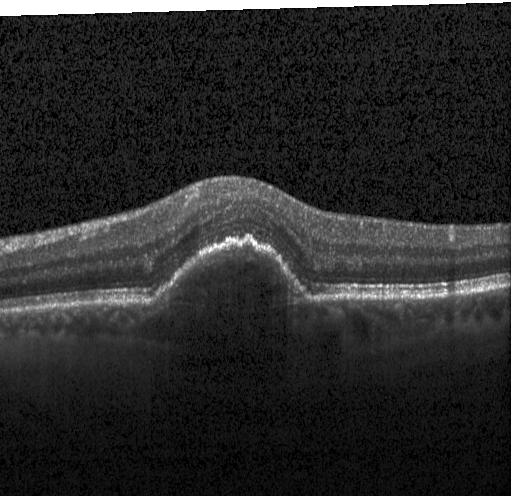

Acquired on a Heidelberg Spectralis · optical coherence tomography scan
The scan shows a choroidal neovascular membrane.